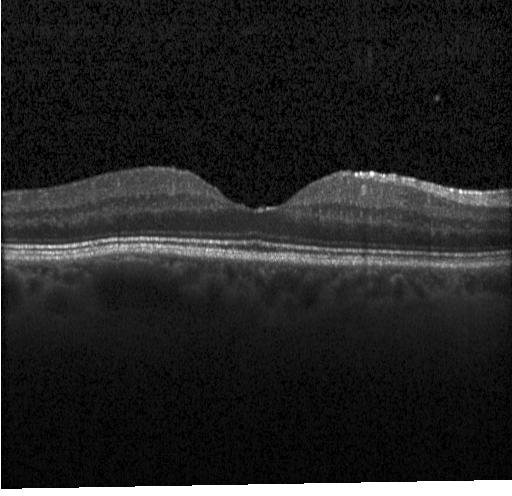 OCT finding: no CNV, no DME, and no drusen.